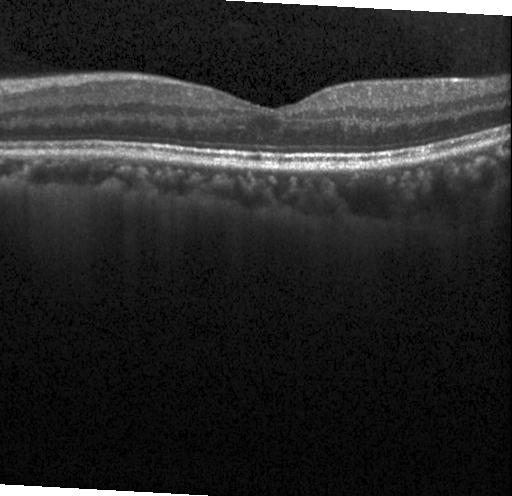

Spectral-domain OCT; OCT line scan
Macular OCT: no evidence of choroidal neovascularization, diabetic macular edema, or drusen.